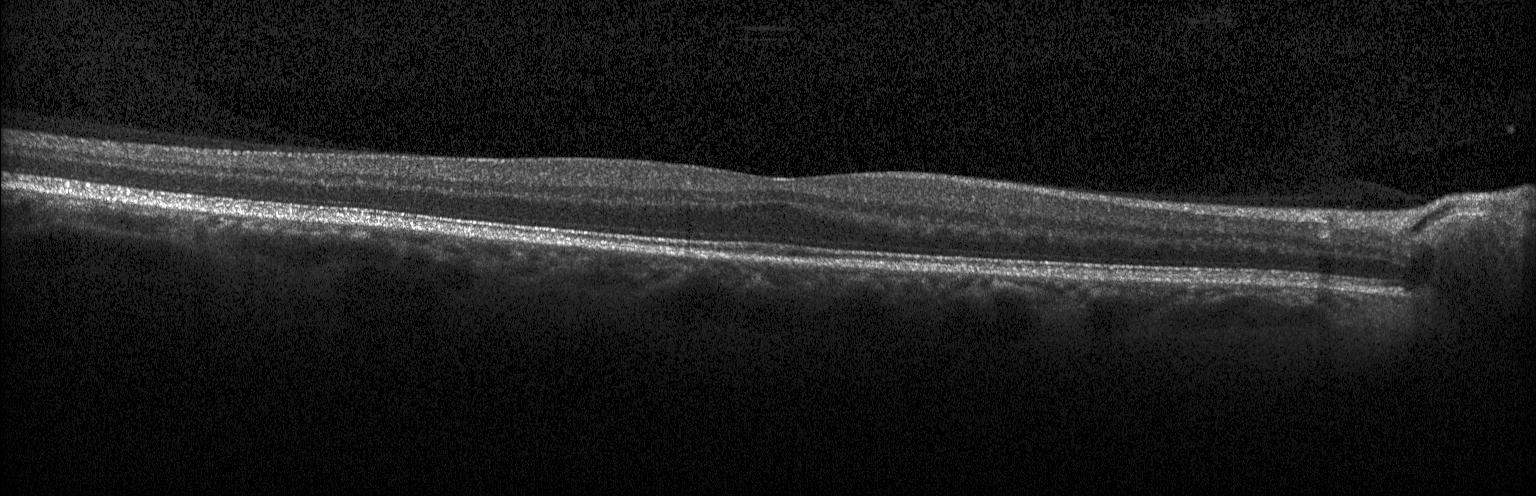
Heidelberg Spectralis OCT system · optical coherence tomography B-scan. Finding: no choroidal neovascularization, no diabetic macular edema, and no drusen.